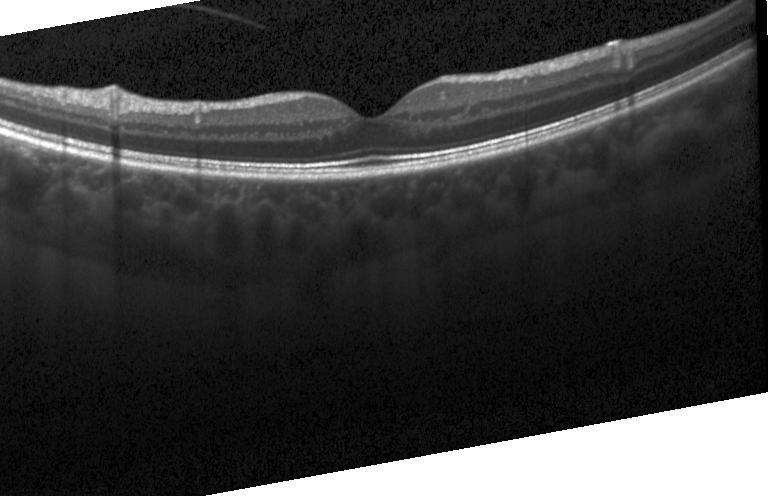

OCT finding: neither choroidal neovascularization, diabetic macular edema, nor drusen.